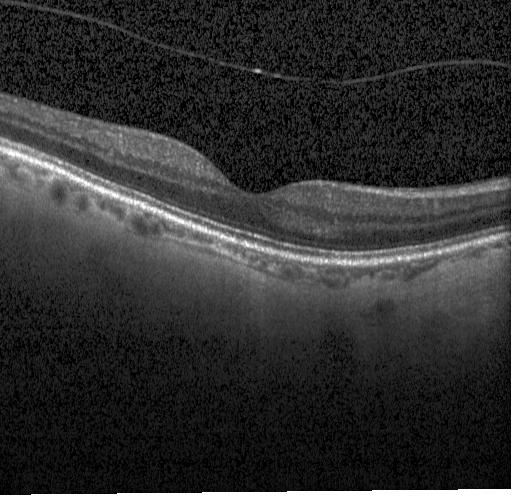

Heidelberg Spectralis OCT system; retinal OCT B-scan. Impression: no CNV, no DME, and no drusen.